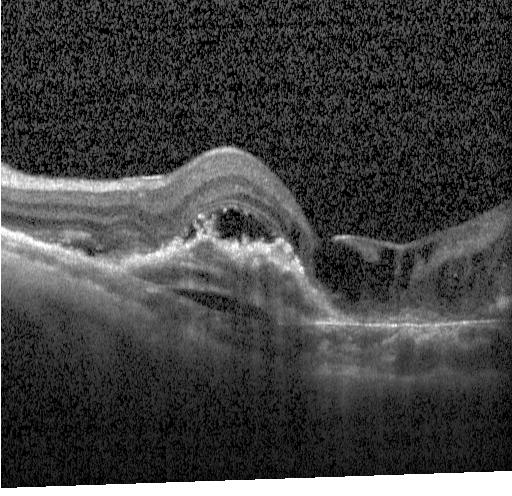 OCT B-scan showing CNV.